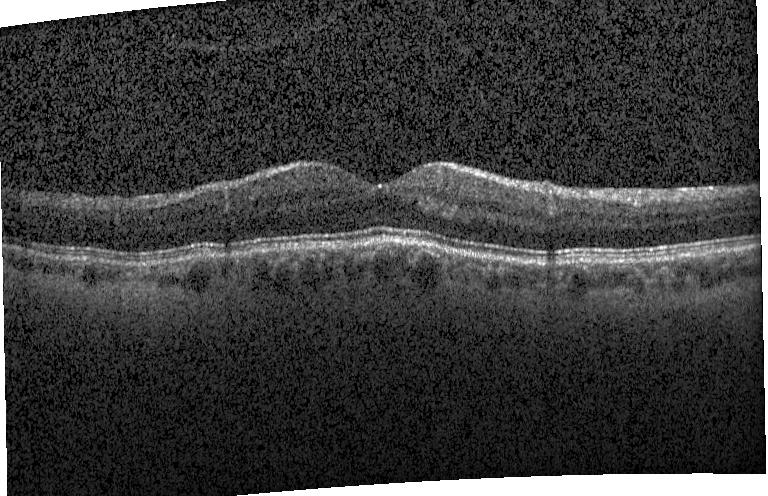

Dx: neither choroidal neovascularization, diabetic macular edema, nor drusen.